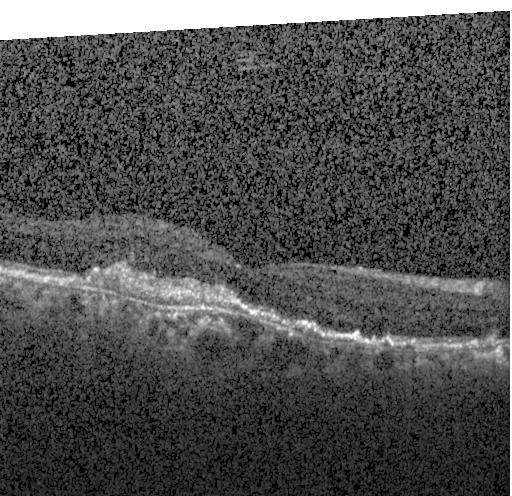

Impression: CNV.